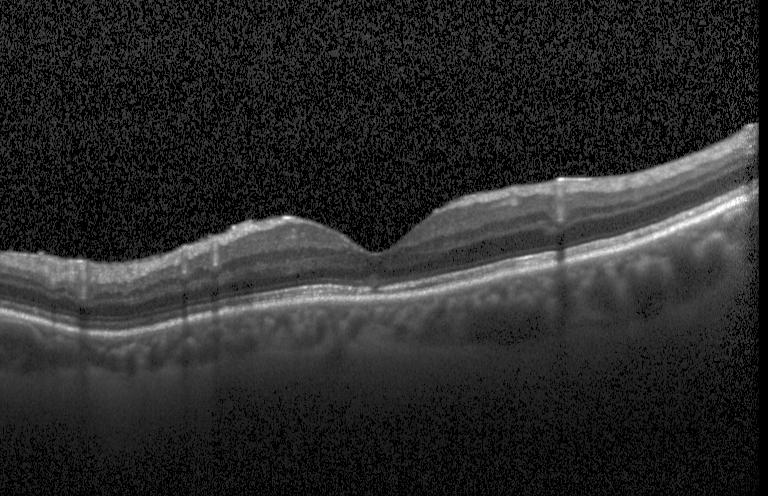 Spectral-domain OCT; OCT B-scan — OCT finding: no choroidal neovascularization, diabetic macular edema, or drusen.